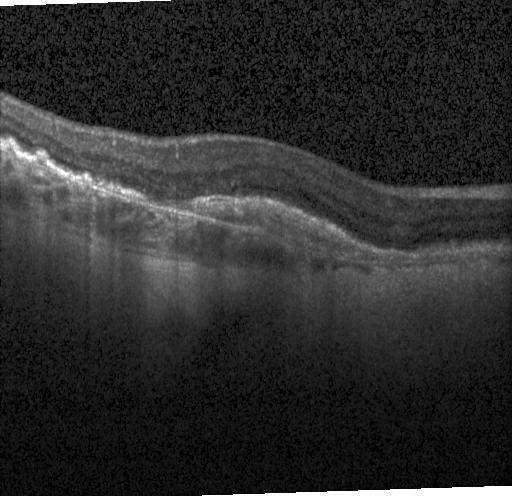
Retinal OCT B-scan
The scan shows a choroidal neovascular membrane.